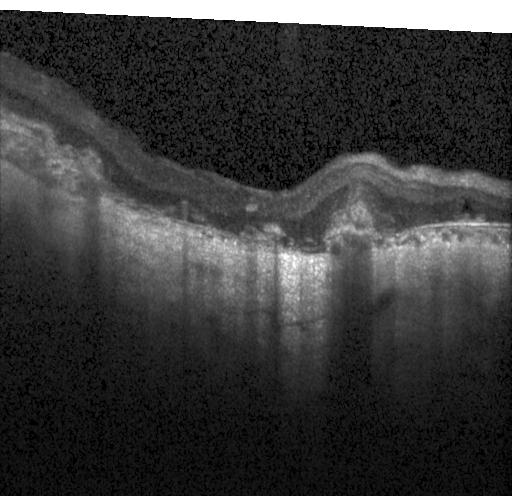 Spectral-domain optical coherence tomography, Heidelberg Spectralis, retinal OCT cross-section, macular scan — Macular OCT: CNV.